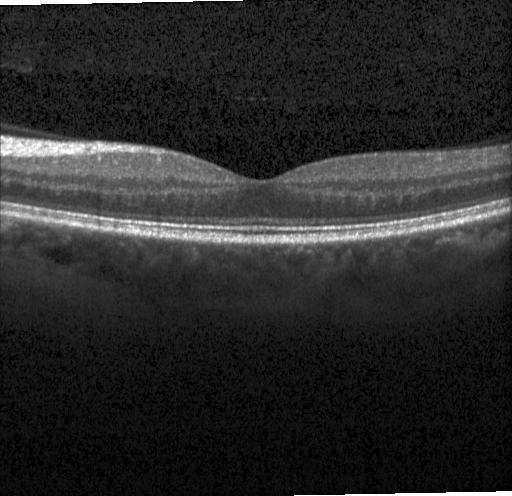

OCT B-scan showing neither choroidal neovascularization, diabetic macular edema, nor drusen.